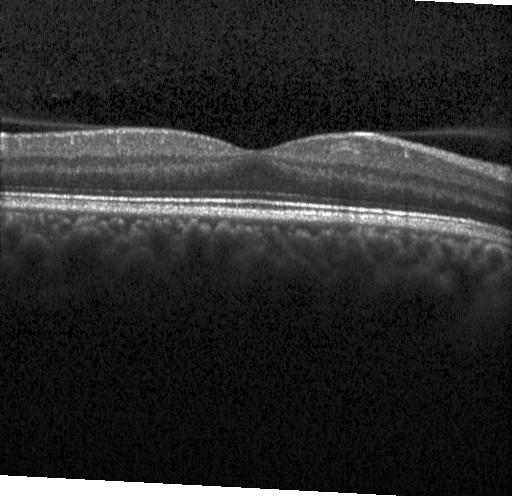

OCT line scan — Macular OCT: no evidence of choroidal neovascularization, diabetic macular edema, or drusen.